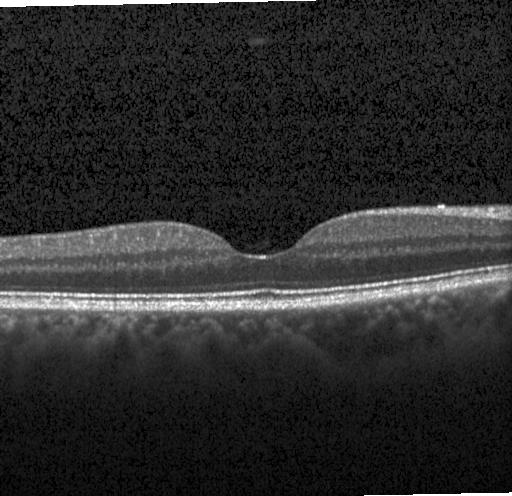
Optical coherence tomography B-scan
Assessment: no CNV, DME, or drusen.